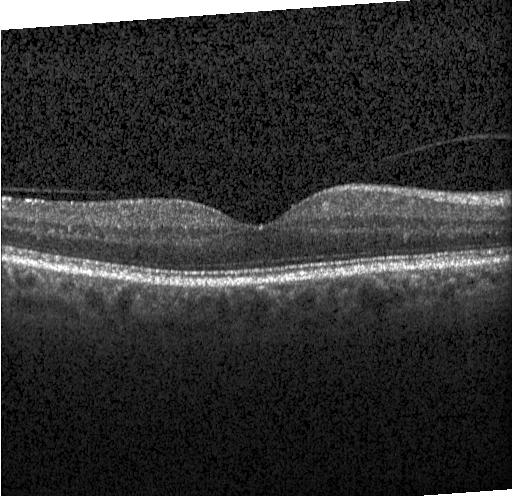
Optical coherence tomography scan, acquired on a Heidelberg Spectralis, macular scan.
Impression: neither CNV, DME, nor drusen.